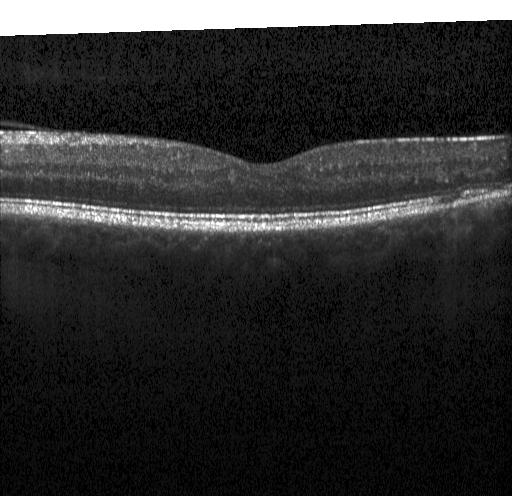 No evidence of CNV, DME, or drusen.